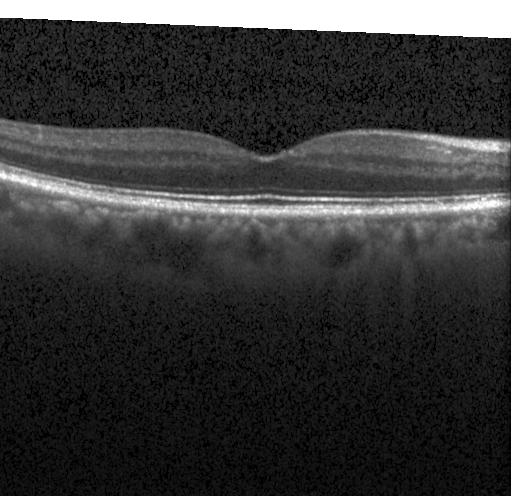 Finding: no choroidal neovascularization, diabetic macular edema, or drusen.